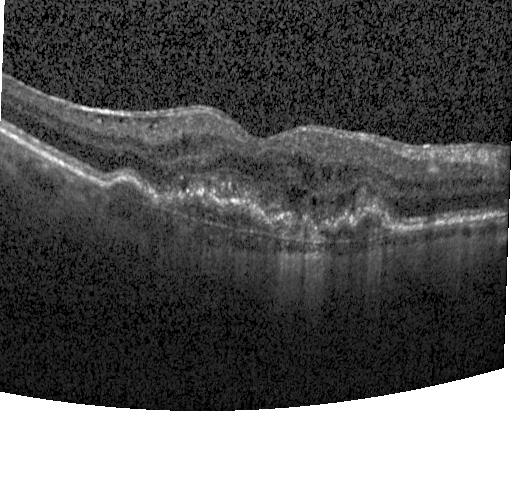 Dx: CNV.